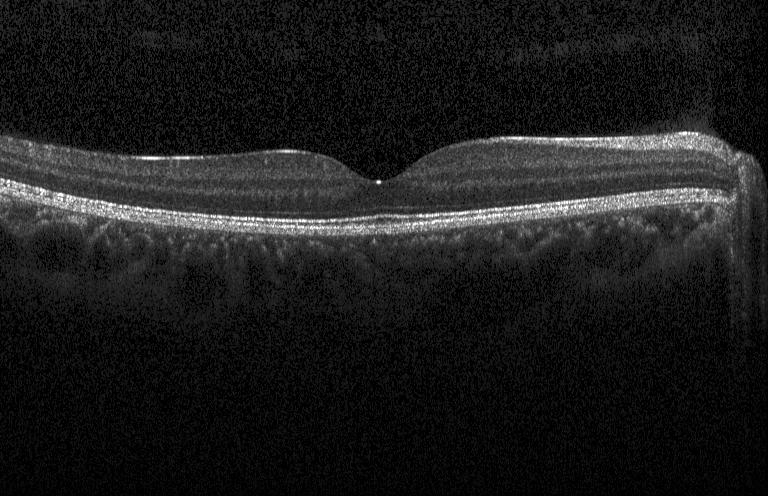 SD-OCT. OCT line scan. Horizontal scan through the fovea. Heidelberg Spectralis OCT system. The scan shows no evidence of choroidal neovascularization, diabetic macular edema, or drusen.